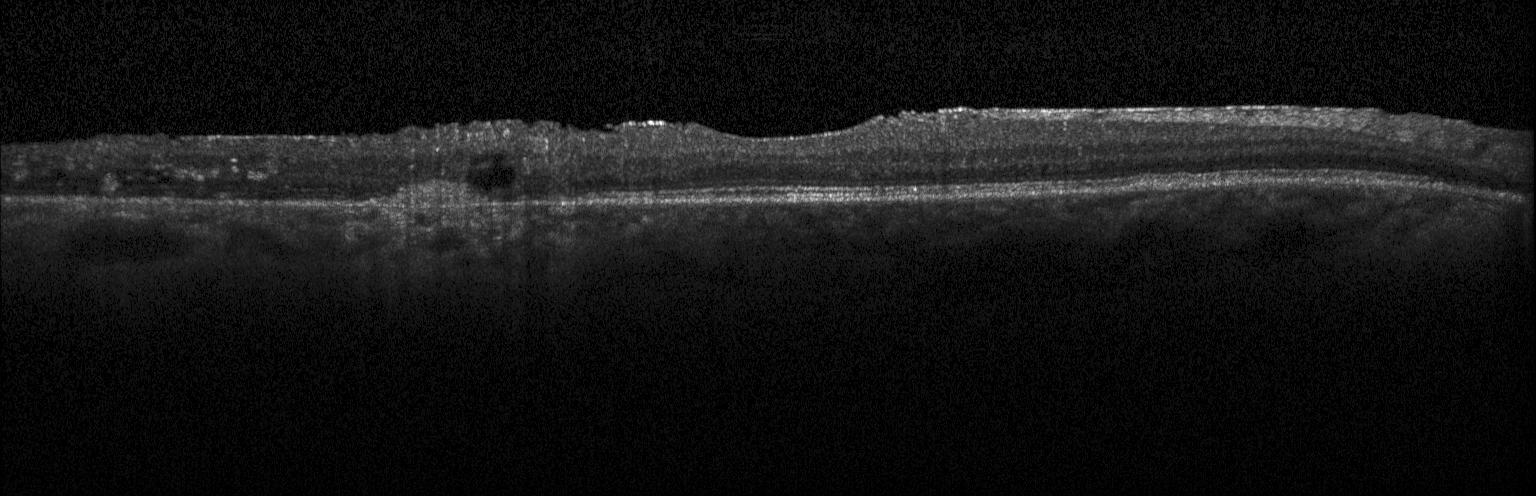
Dx: a choroidal neovascular membrane.